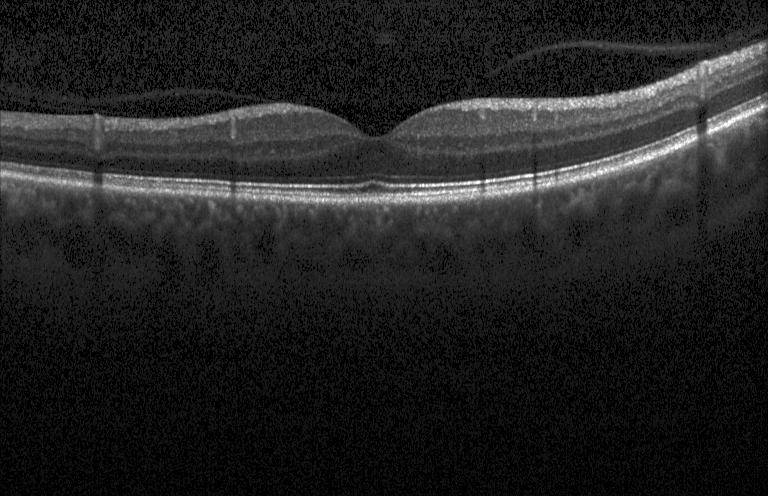
OCT line scan. Spectral-domain OCT
Diagnosis: no choroidal neovascularization, diabetic macular edema, or drusen.